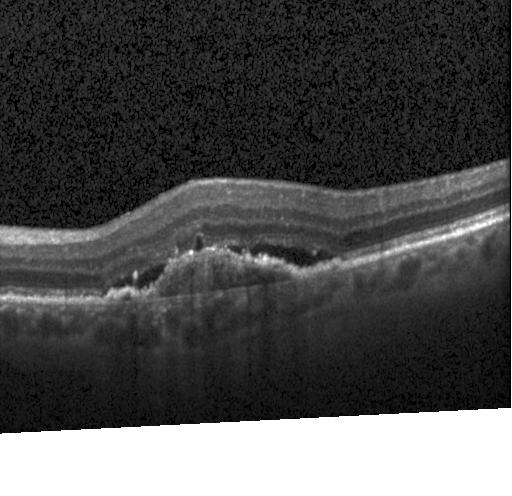

Retinal OCT cross-section showing a choroidal neovascular membrane.